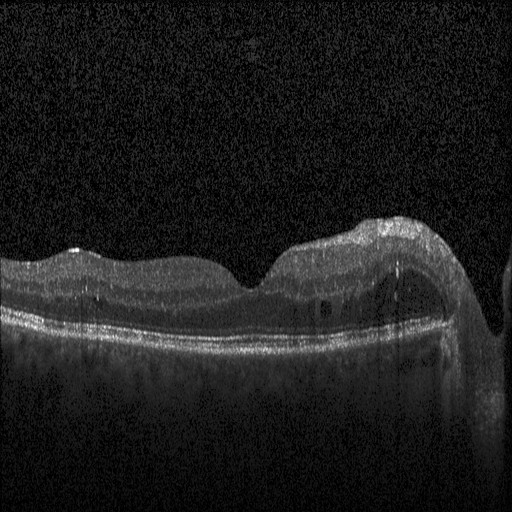

OCT scan showing diabetic macular edema.